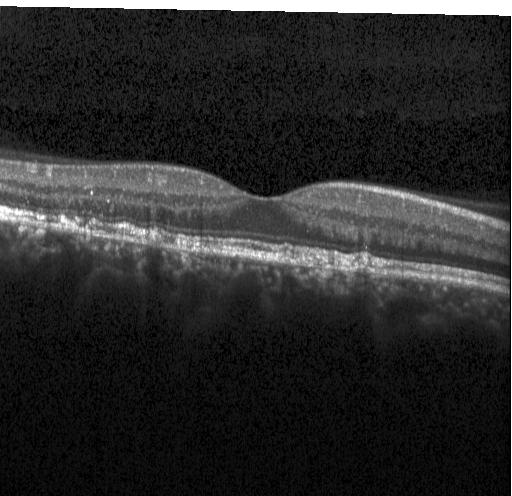

Optical coherence tomography B-scan, centered on the fovea.
Diagnosis: drusen.